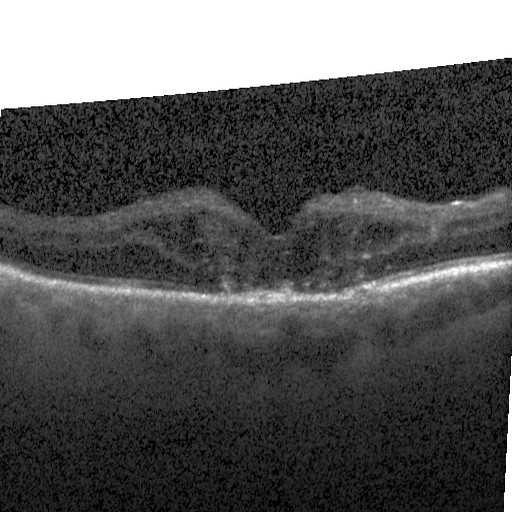

Macular OCT: diabetic macular edema (DME).